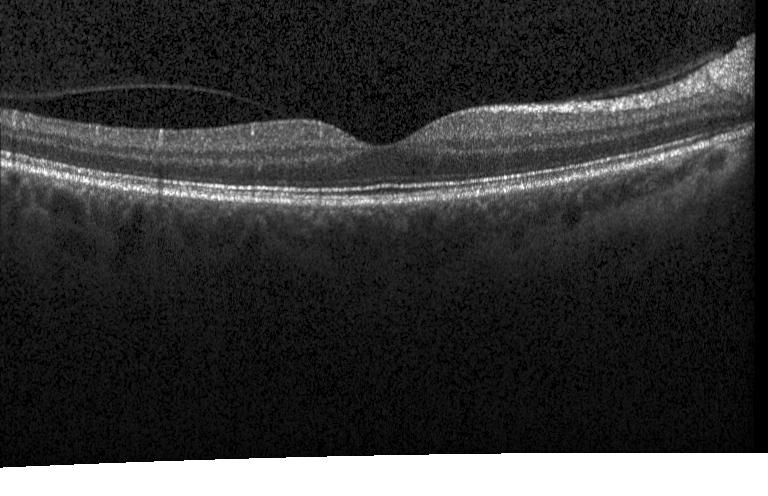 Centered on the fovea · OCT line scan · SD-OCT
Finding: no choroidal neovascularization, no diabetic macular edema, and no drusen.